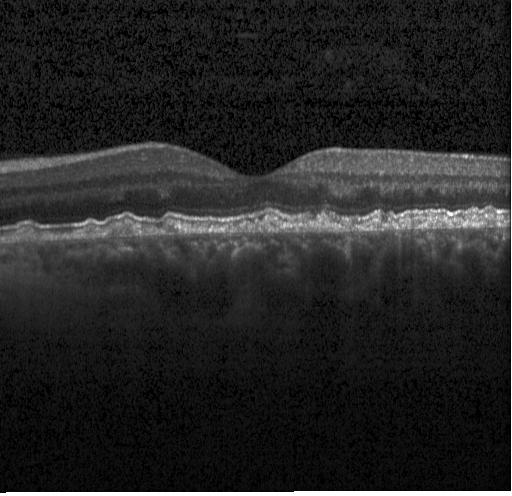

OCT scan showing multiple drusen.